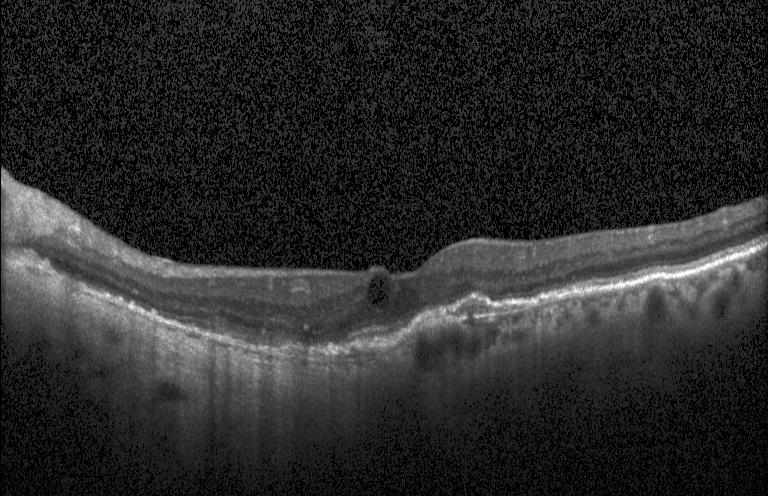

SD-OCT; acquired on a Heidelberg Spectralis; retinal OCT B-scan. Finding: a choroidal neovascular membrane.